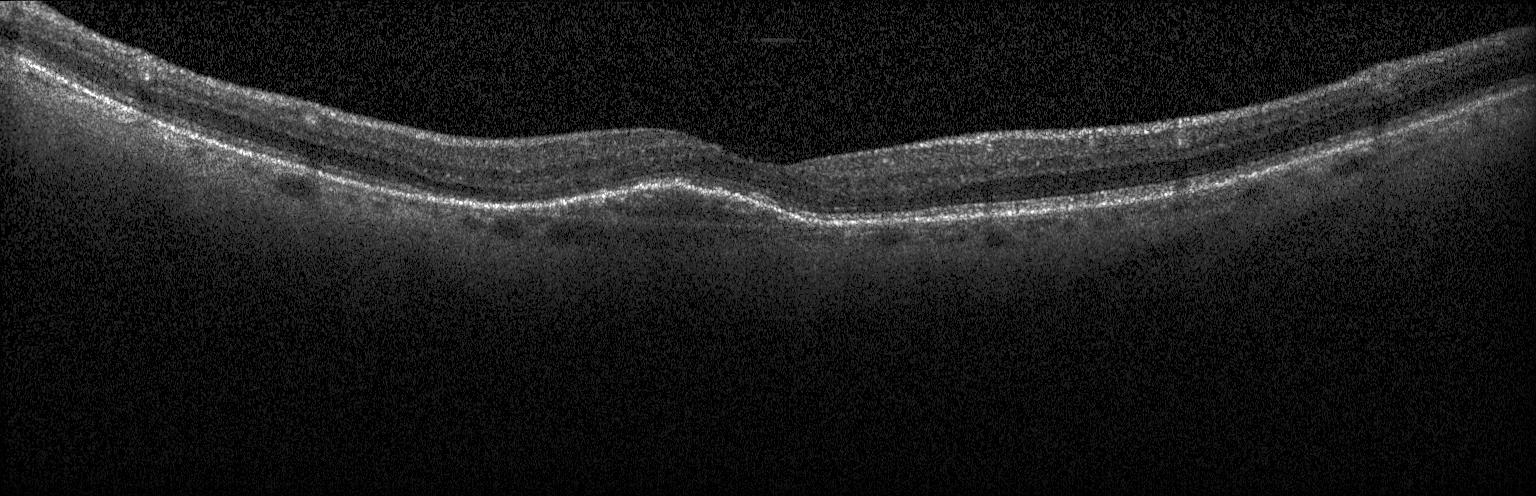

Choroidal neovascularization (CNV).